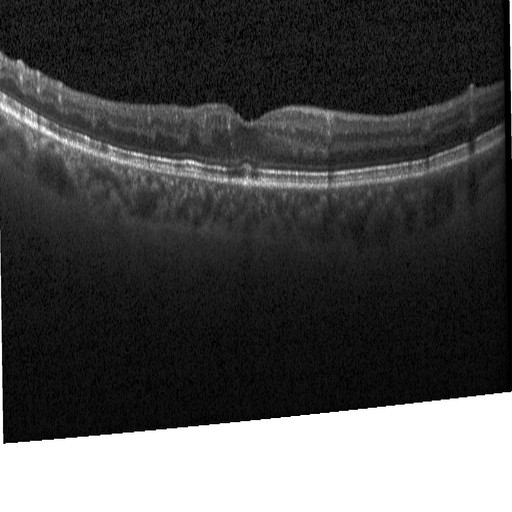
Macular OCT: diabetic macular edema (DME).